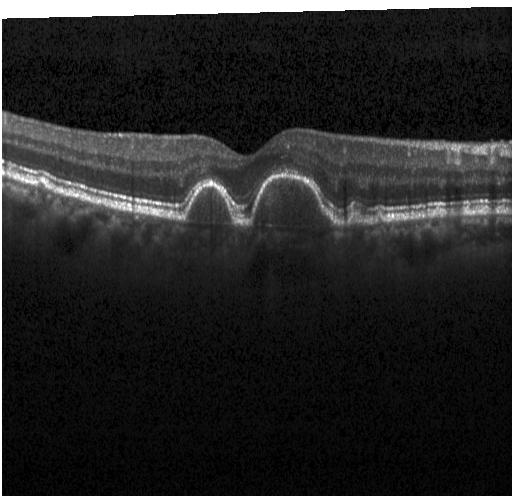

Optical coherence tomography B-scan; horizontal scan through the fovea — This B-scan demonstrates multiple drusen.